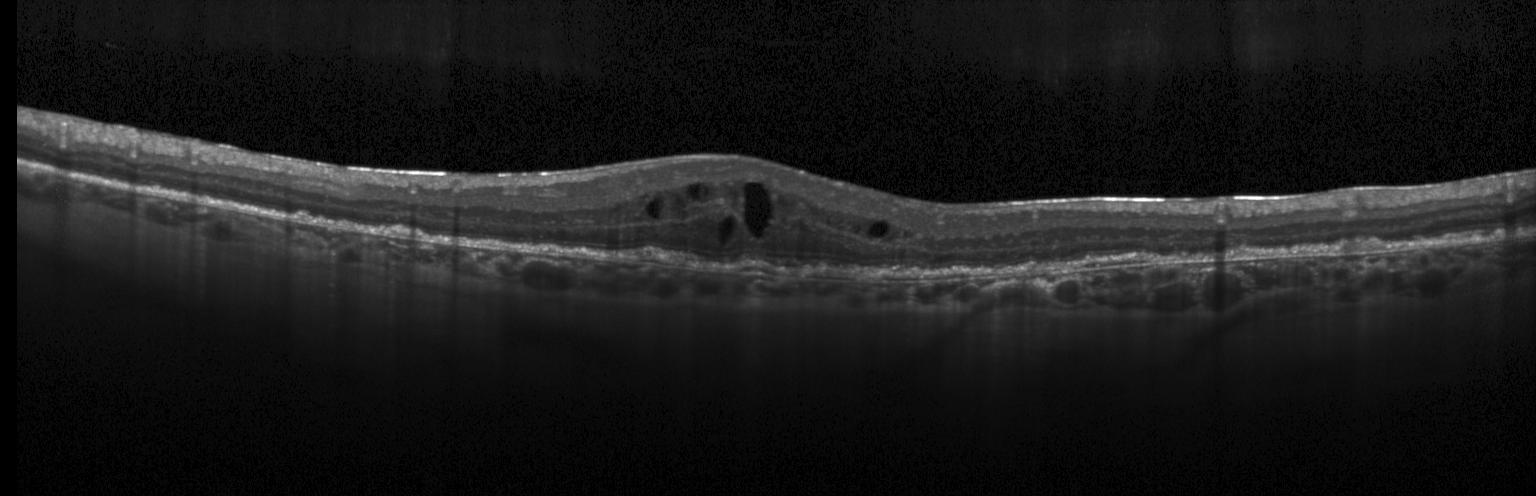 OCT line scan; fovea-centered; acquired on a Heidelberg Spectralis; spectral-domain OCT — This B-scan demonstrates choroidal neovascularization.